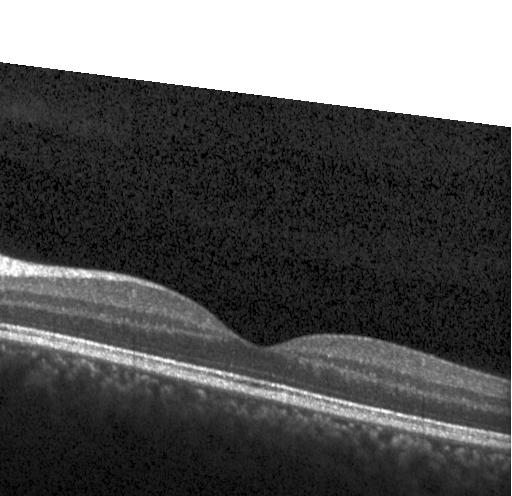 Impression: no choroidal neovascularization, no diabetic macular edema, and no drusen.